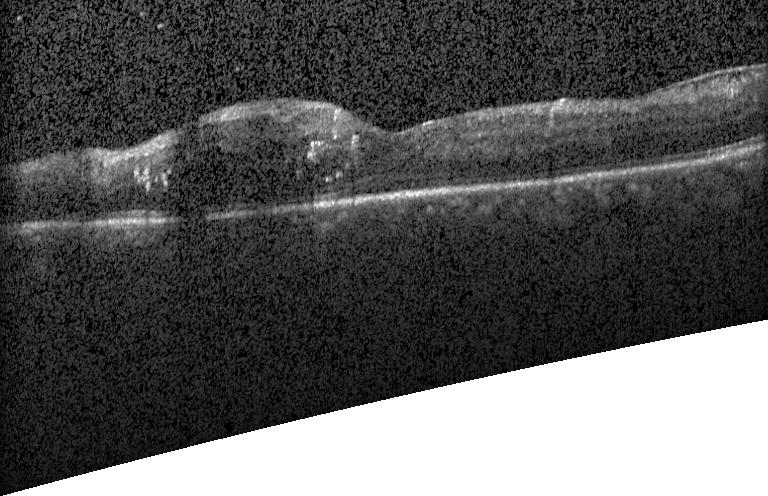

Diagnosis: diabetic macular edema.